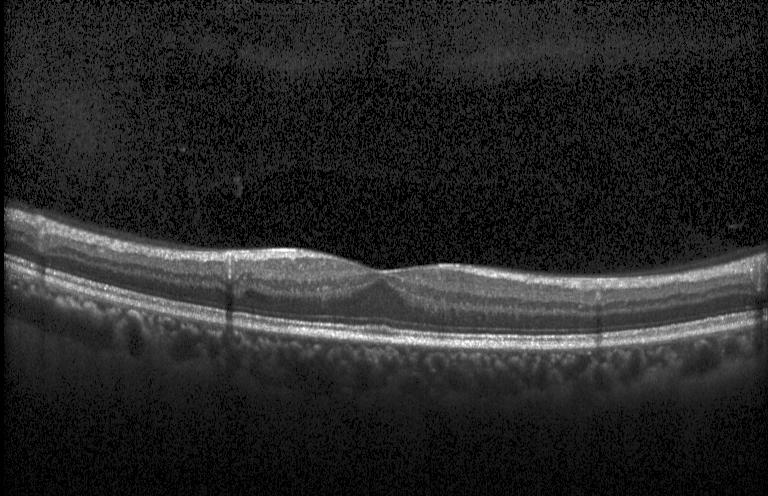 Retinal OCT cross-section showing no CNV, no DME, and no drusen.